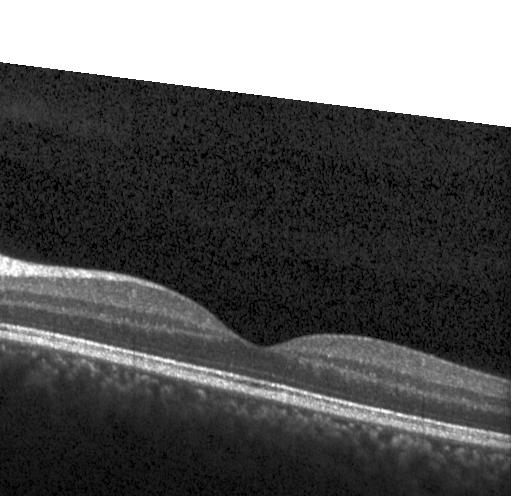
Retinal OCT B-scan, Heidelberg Spectralis — Macular OCT: no evidence of choroidal neovascularization, diabetic macular edema, or drusen.